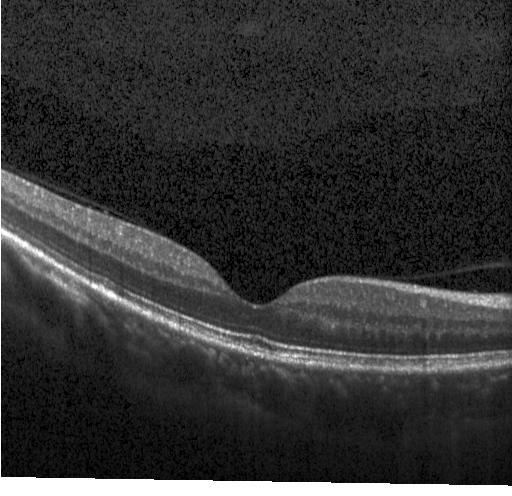

Spectral-domain OCT · horizontal scan through the fovea · retinal OCT B-scan — Impression: no choroidal neovascularization, no diabetic macular edema, and no drusen.